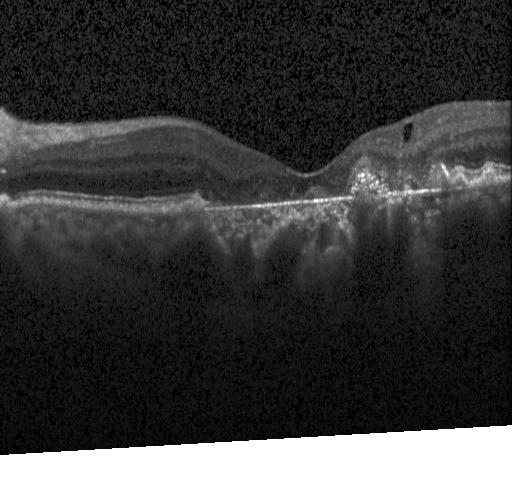
Spectral-domain OCT B-scan: a choroidal neovascular membrane.